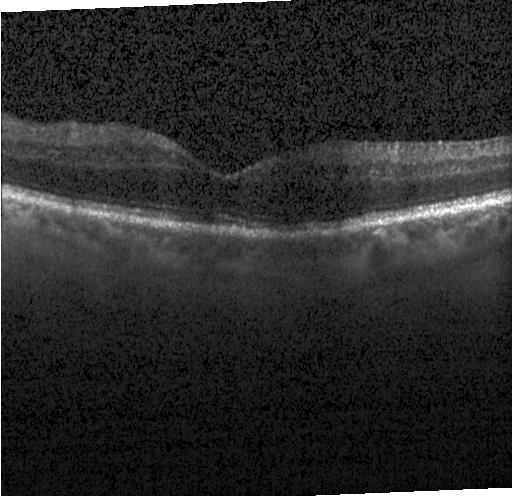

Macular OCT: no choroidal neovascularization, no diabetic macular edema, and no drusen.